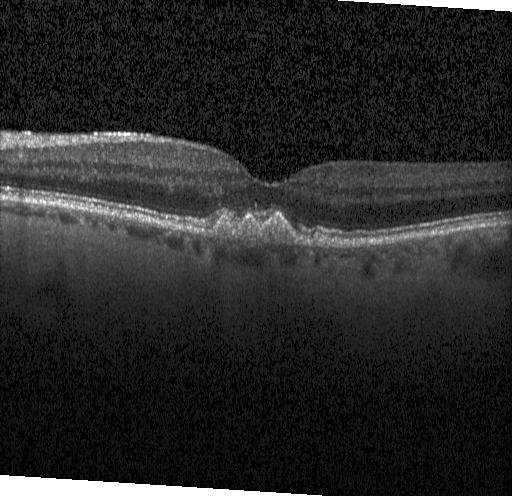

Assessment: sub-RPE drusenoid deposits.